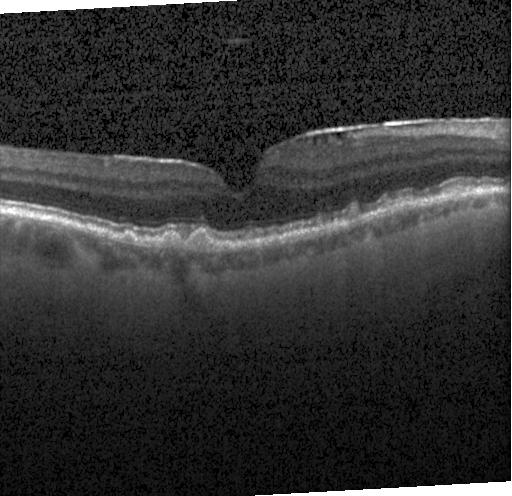 Dx: multiple drusen.